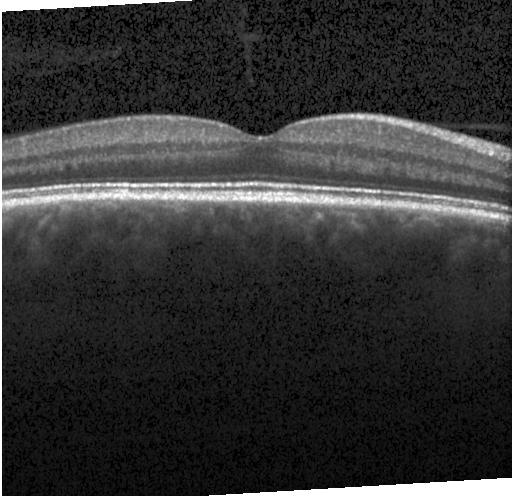
Optical coherence tomography B-scan. Impression: no CNV, no DME, and no drusen.